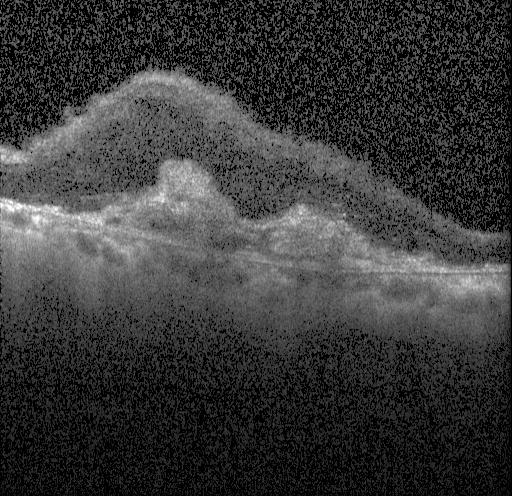 Retinal OCT cross-section showing choroidal neovascularization (CNV).